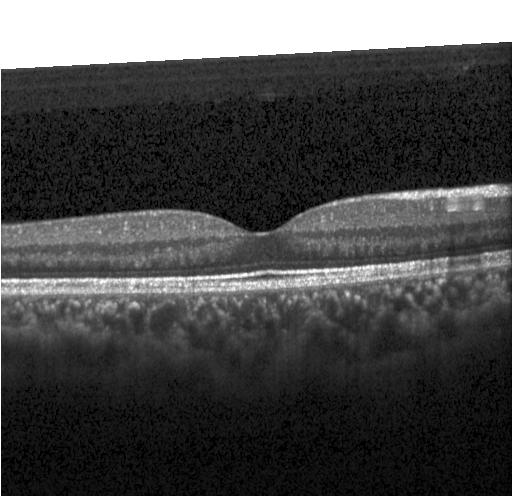

Macular OCT demonstrating no choroidal neovascularization, no diabetic macular edema, and no drusen.